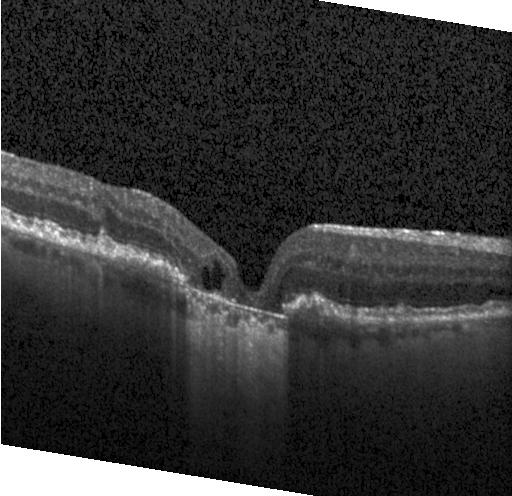

Retinal OCT B-scan — Finding: a choroidal neovascular membrane.